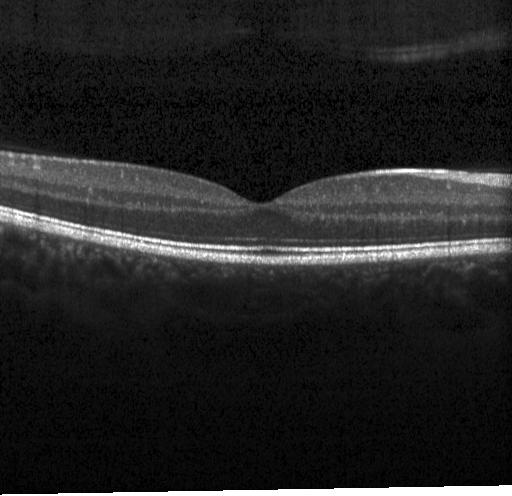 Optical coherence tomography scan, fovea-centered, spectral-domain OCT, Heidelberg Spectralis OCT system — Assessment: no choroidal neovascularization, diabetic macular edema, or drusen.